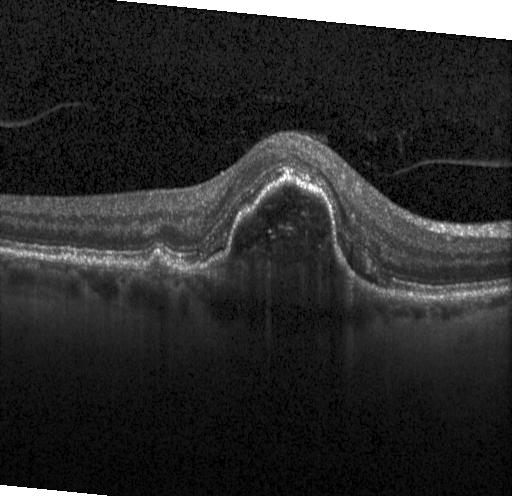
Retinal OCT cross-section. This B-scan demonstrates CNV.